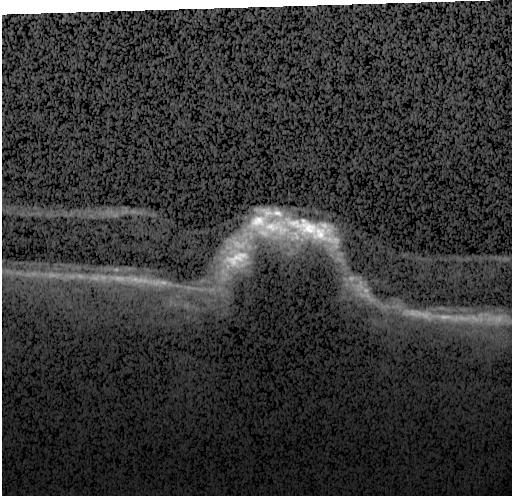
Diagnosis: choroidal neovascularization (CNV).